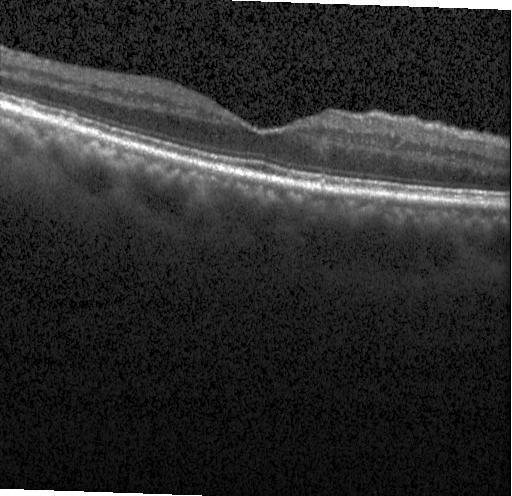 Heidelberg Spectralis, retinal OCT cross-section, fovea-centered. This B-scan demonstrates no CNV, no DME, and no drusen.